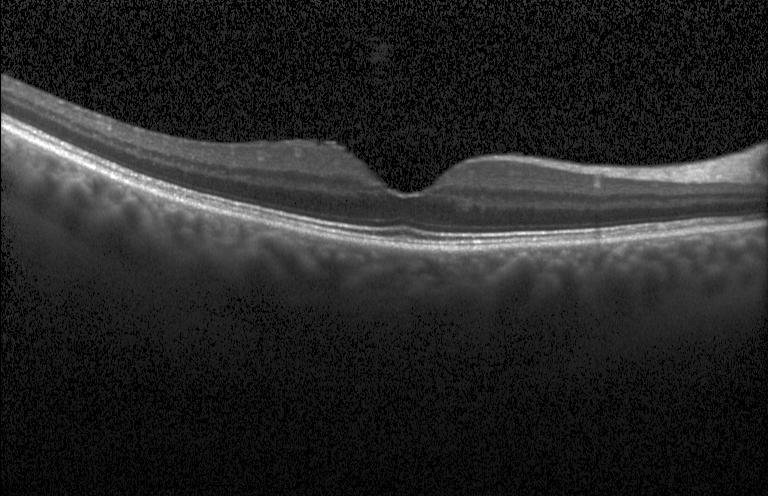 Instrument: Heidelberg Spectralis · horizontal scan through the fovea · retinal OCT cross-section — Finding: no CNV, DME, or drusen.